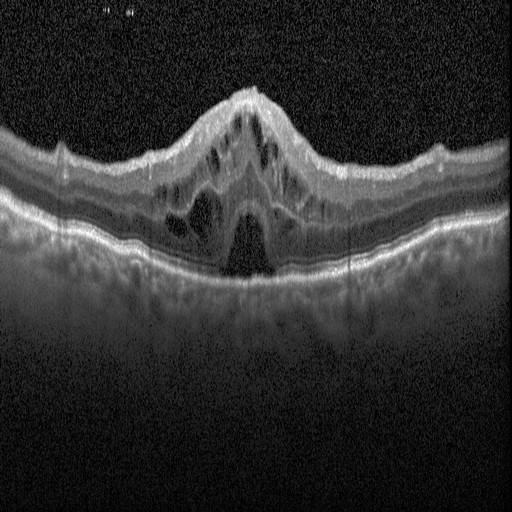 Assessment: diabetic macular edema (DME).